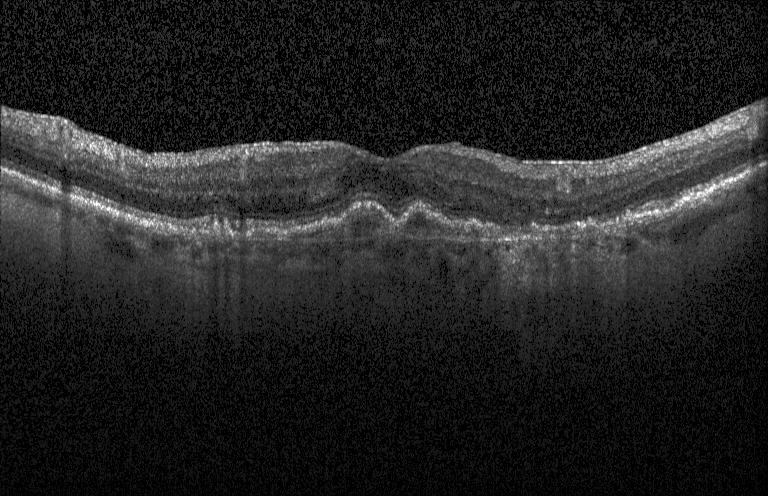 Spectral-domain OCT · Heidelberg Spectralis · through the macula · OCT line scan.
OCT finding: a choroidal neovascular membrane.